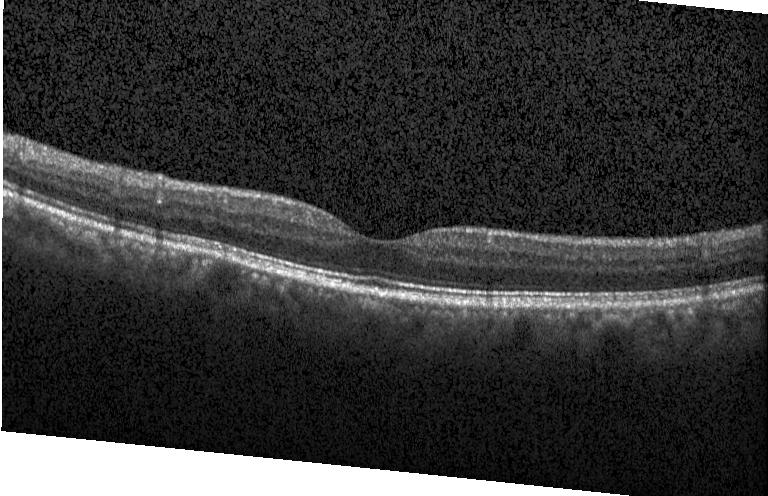 Impression: no choroidal neovascularization, diabetic macular edema, or drusen.